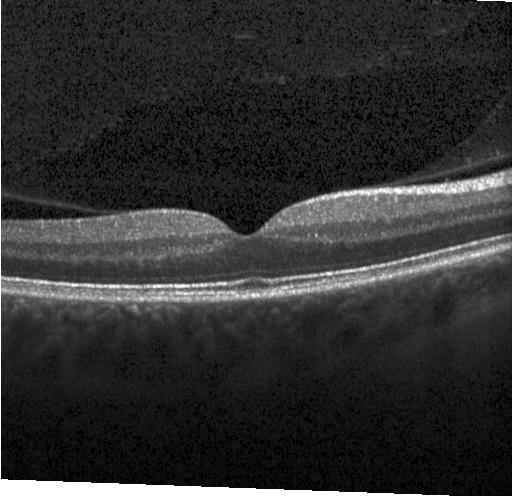
Diagnosis: no evidence of CNV, DME, or drusen.